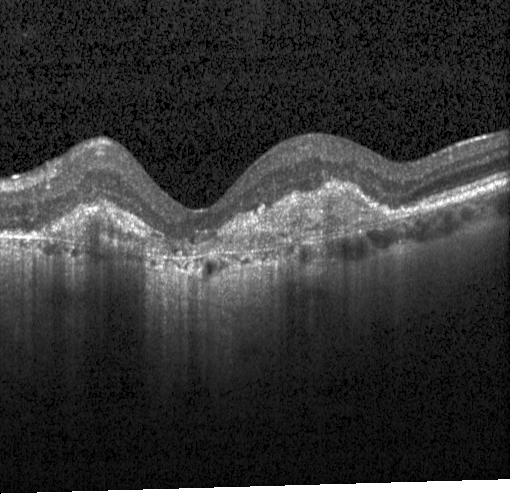
Impression: CNV.